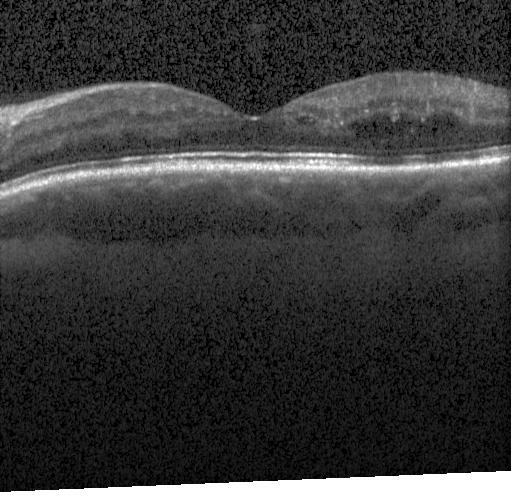 OCT line scan. Acquired on a Heidelberg Spectralis — Impression: diabetic macular edema (DME).